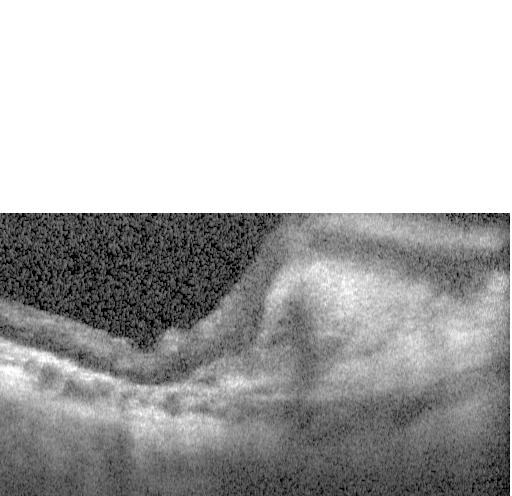 Retinal OCT cross-section — Impression: CNV.